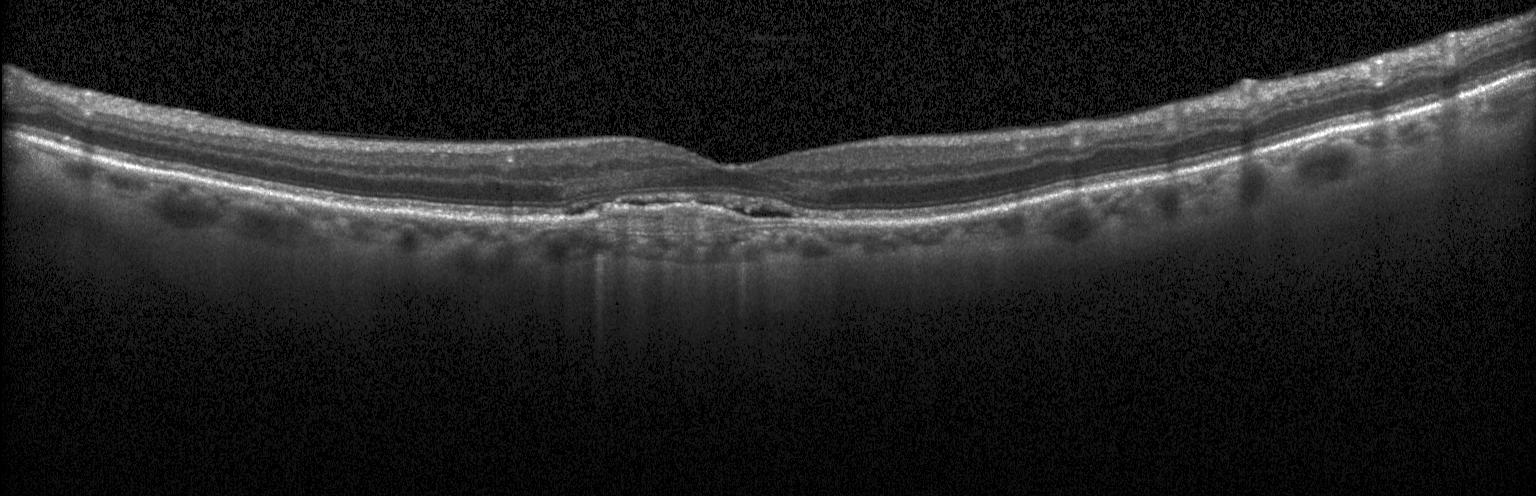

Retinal OCT cross-section
Diagnosis: a choroidal neovascular membrane.